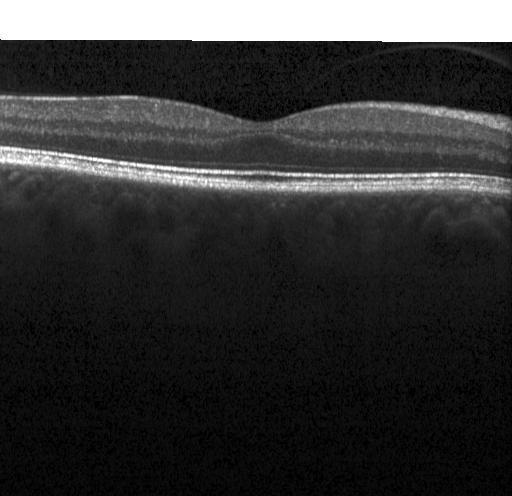

OCT line scan. Spectral-domain OCT. Through the macula.
OCT finding: no choroidal neovascularization, no diabetic macular edema, and no drusen.